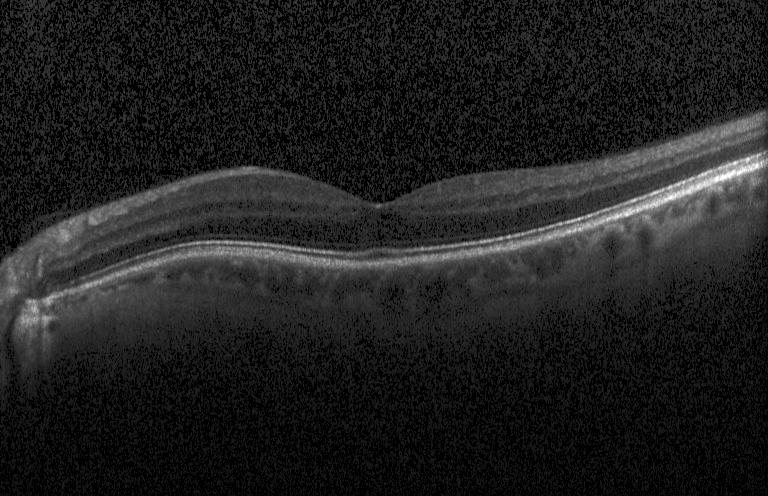
Through the macula. Optical coherence tomography B-scan.
Dx: neither CNV, DME, nor drusen.